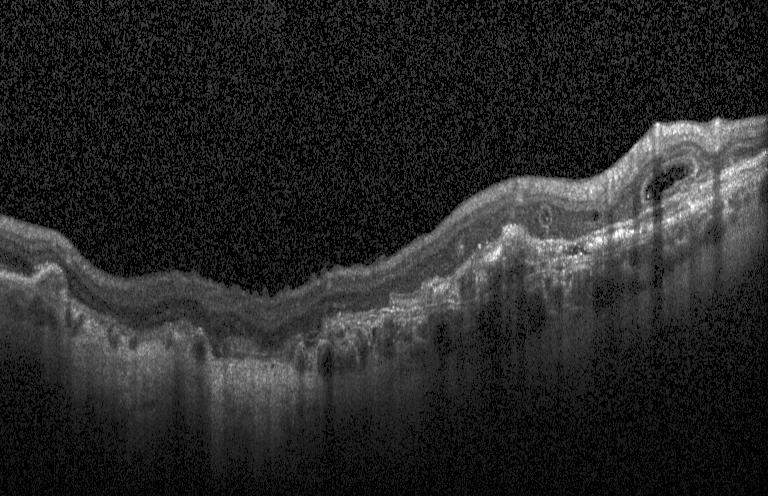
Finding: choroidal neovascularization (CNV).